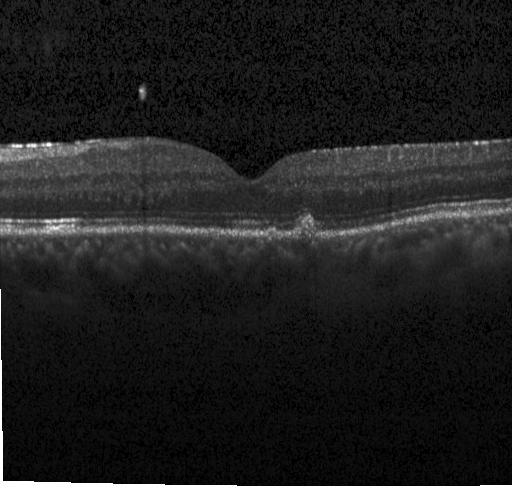
Multiple drusen.